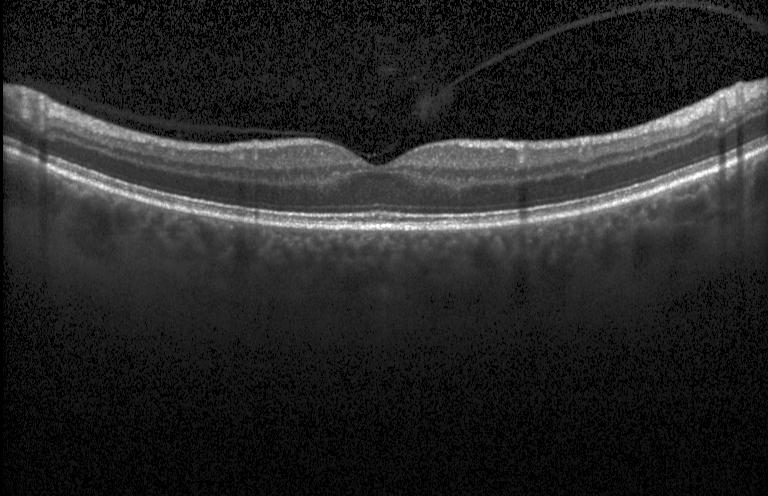

Diagnosis: no evidence of choroidal neovascularization, diabetic macular edema, or drusen.